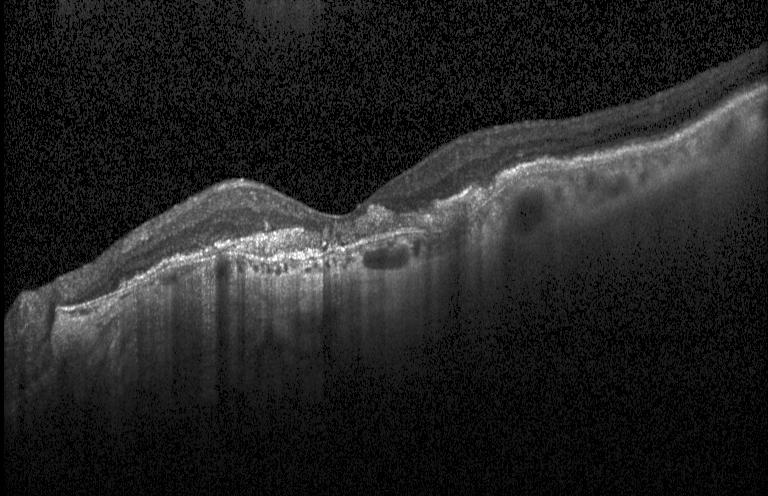
Retinal OCT cross-section showing CNV.